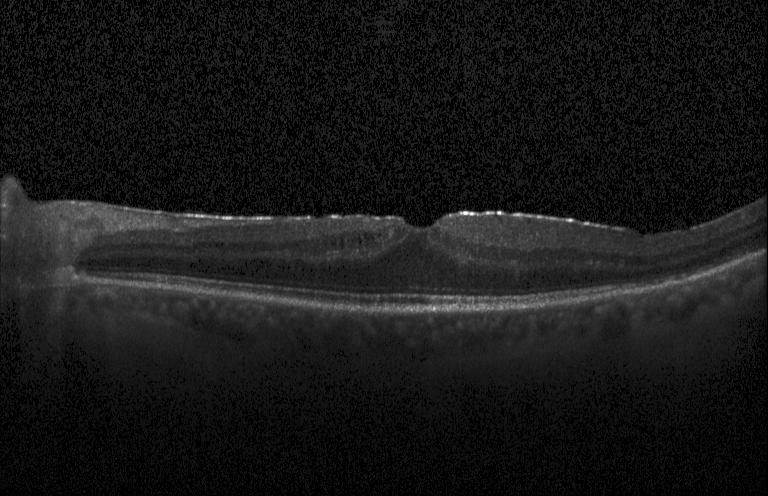 OCT B-scan · spectral-domain OCT · macular scan.
The scan shows diabetic macular edema.